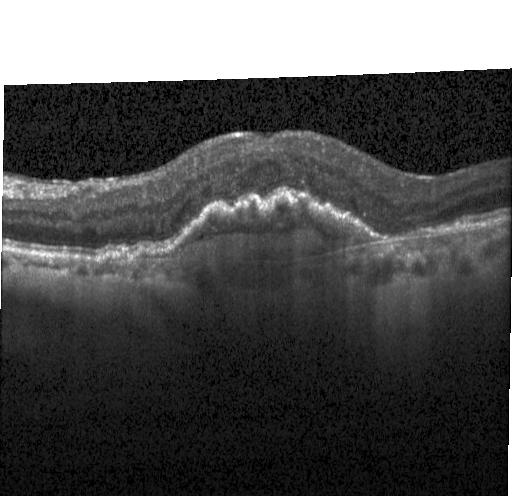
Diagnosis: a choroidal neovascular membrane.